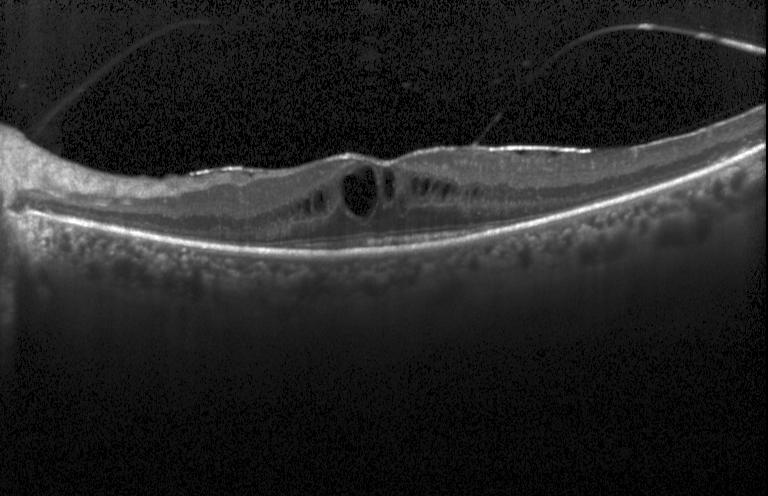
Fovea-centered. Optical coherence tomography scan.
The scan shows diabetic macular edema.